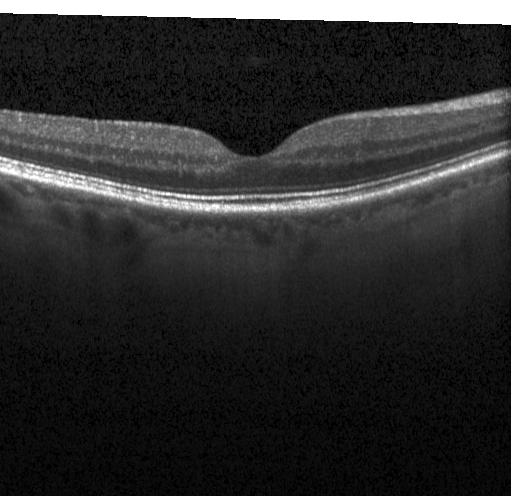 Diagnosis: no choroidal neovascularization, no diabetic macular edema, and no drusen.